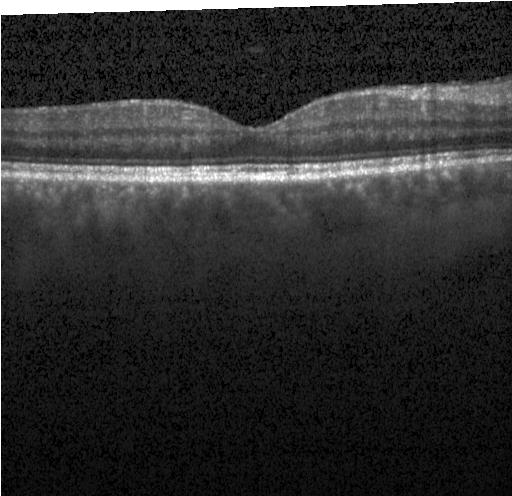 OCT B-scan, spectral-domain optical coherence tomography, Heidelberg Spectralis OCT system, horizontal scan through the fovea
Finding: no CNV, DME, or drusen.